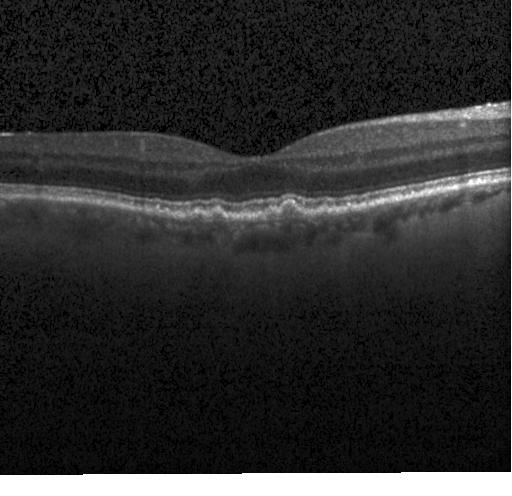
SD-OCT; OCT B-scan — Macular OCT: sub-RPE drusenoid deposits.